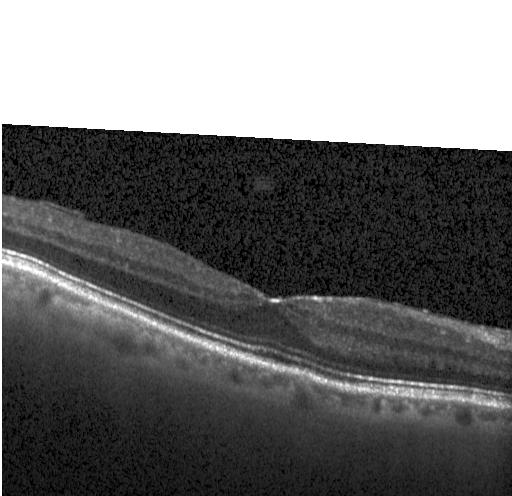
Retinal OCT cross-section; SD-OCT; through the macula; instrument: Heidelberg Spectralis
Dx: no evidence of choroidal neovascularization, diabetic macular edema, or drusen.